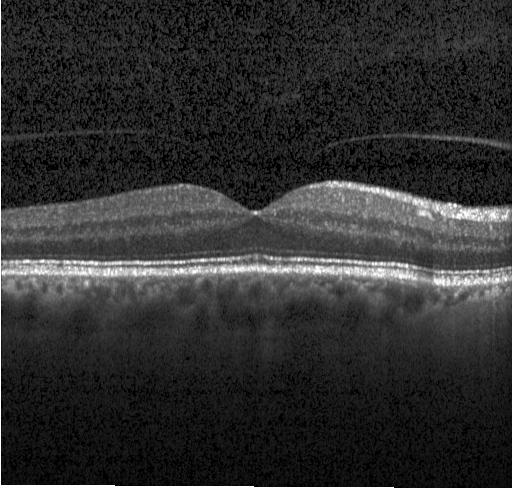 SD-OCT. Heidelberg Spectralis OCT system. Retinal OCT cross-section.
No choroidal neovascularization, no diabetic macular edema, and no drusen.